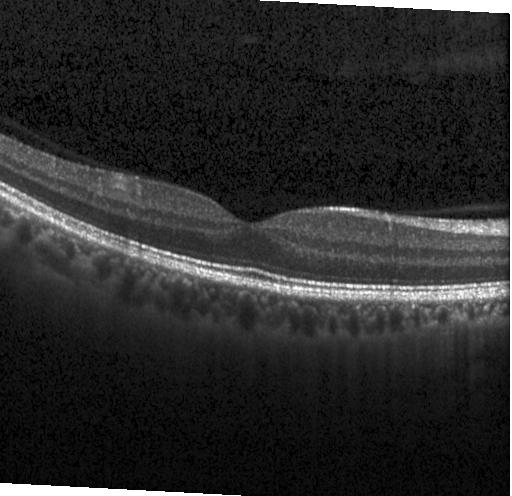 Spectral-domain optical coherence tomography · optical coherence tomography scan.
Assessment: no evidence of CNV, DME, or drusen.